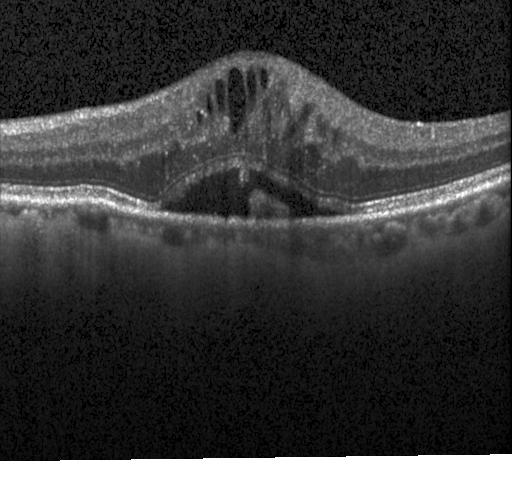
OCT B-scan
Diagnosis: diabetic macular edema.